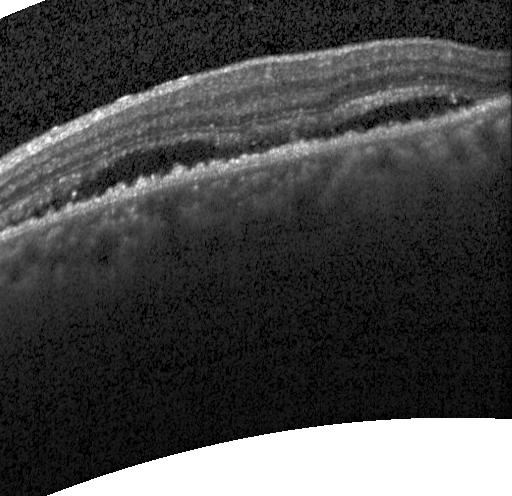 Horizontal scan through the fovea. Optical coherence tomography B-scan. Spectral-domain OCT.
Impression: choroidal neovascularization (CNV).